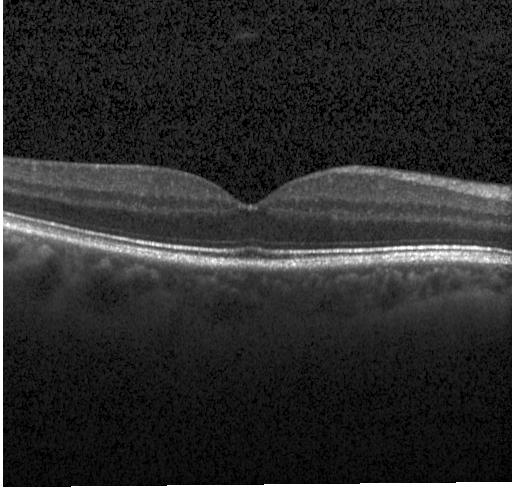

The scan shows no evidence of choroidal neovascularization, diabetic macular edema, or drusen.